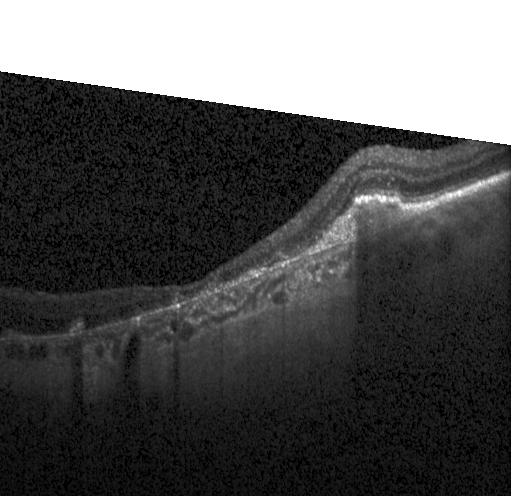
OCT line scan. Macular scan. OCT finding: choroidal neovascularization (CNV).